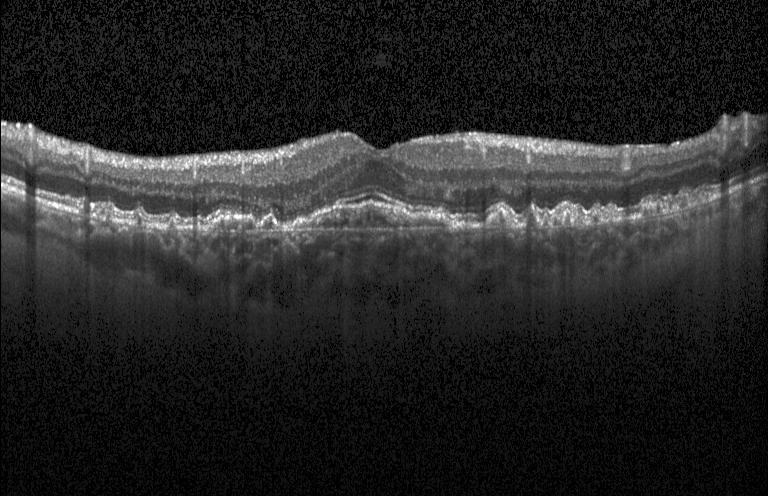

The scan shows choroidal neovascularization (CNV).